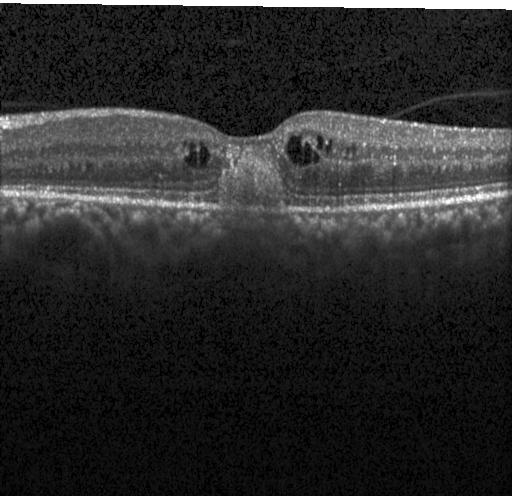 Spectral-domain optical coherence tomography, optical coherence tomography scan.
Impression: a choroidal neovascular membrane.